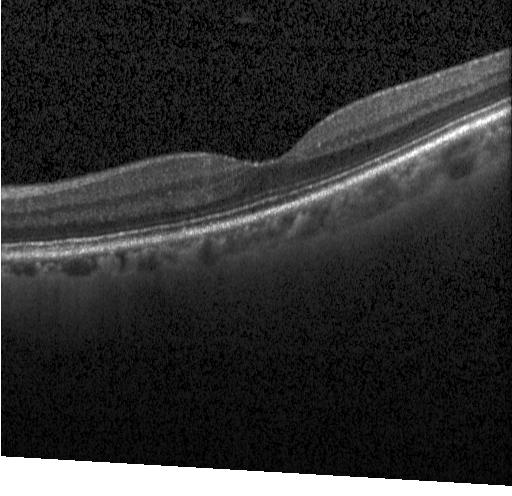
Spectral-domain optical coherence tomography · OCT B-scan · fovea-centered.
Macular OCT: no evidence of CNV, DME, or drusen.